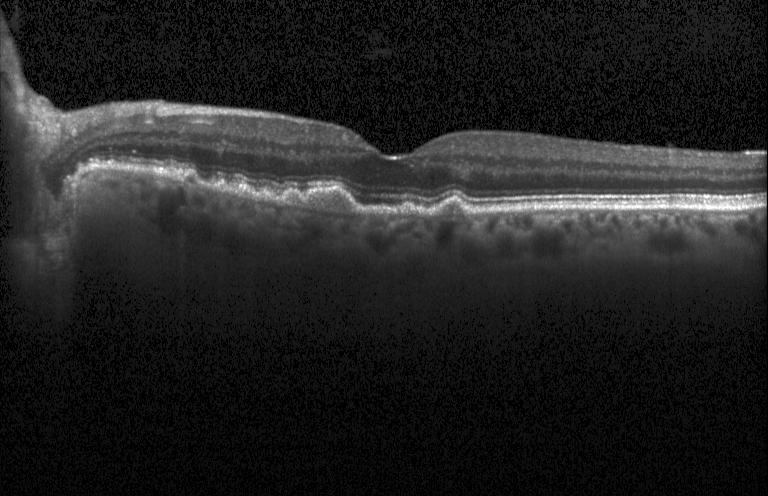
OCT B-scan · centered on the fovea — Diagnosis: sub-RPE drusenoid deposits.